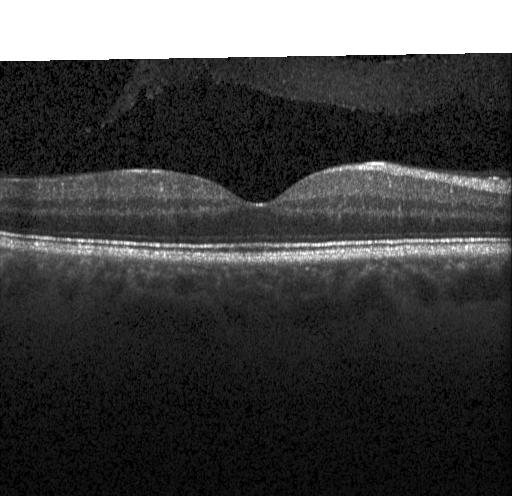 Macular OCT demonstrating no choroidal neovascularization, no diabetic macular edema, and no drusen.